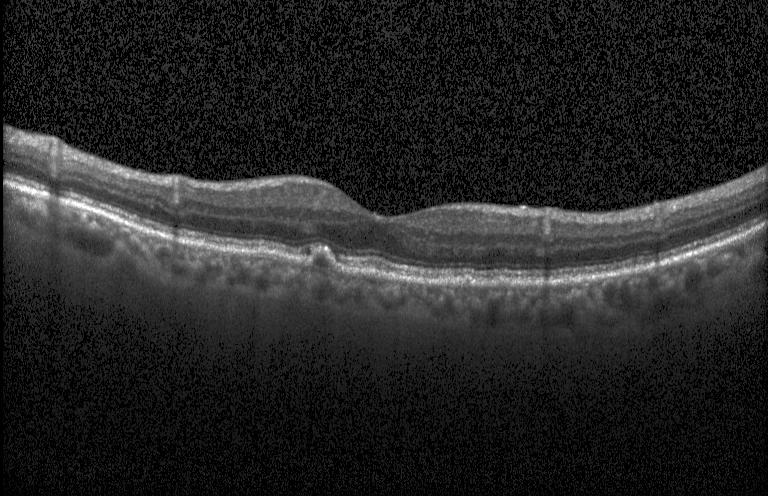
Finding: sub-RPE drusenoid deposits.